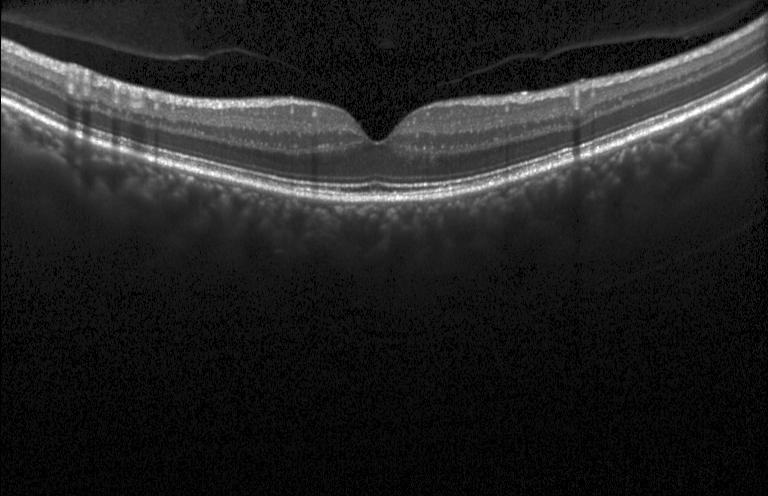
Spectral-domain OCT, macular scan, OCT line scan
Macular OCT: no evidence of choroidal neovascularization, diabetic macular edema, or drusen.